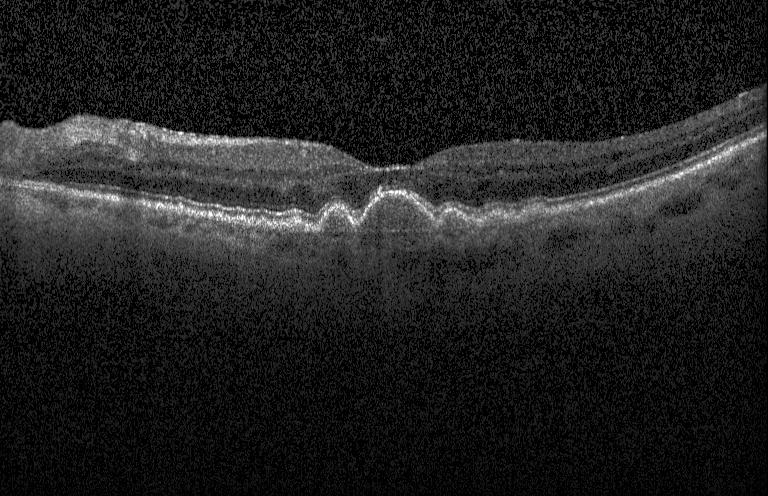

Optical coherence tomography B-scan; SD-OCT.
Assessment: multiple drusen.